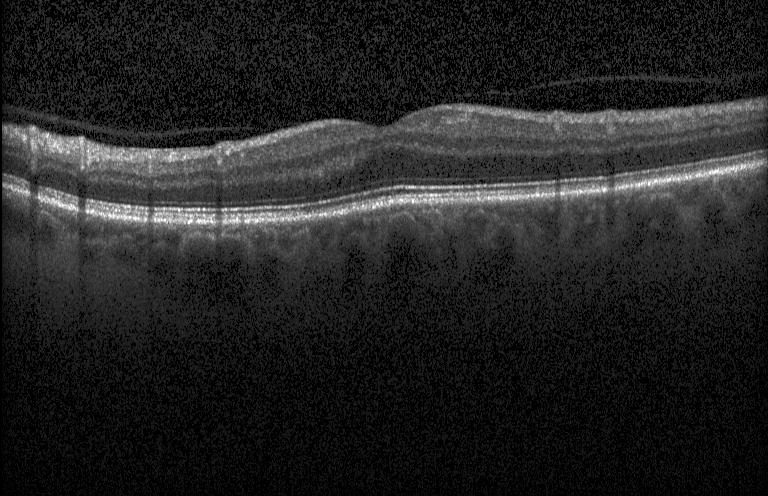 Dx: neither CNV, DME, nor drusen.